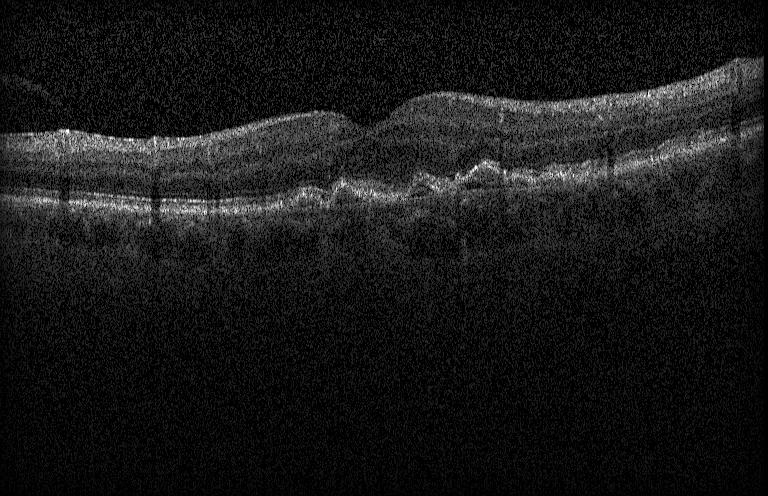
Optical coherence tomography B-scan, Heidelberg Spectralis OCT system, centered on the fovea — Dx: multiple drusen.